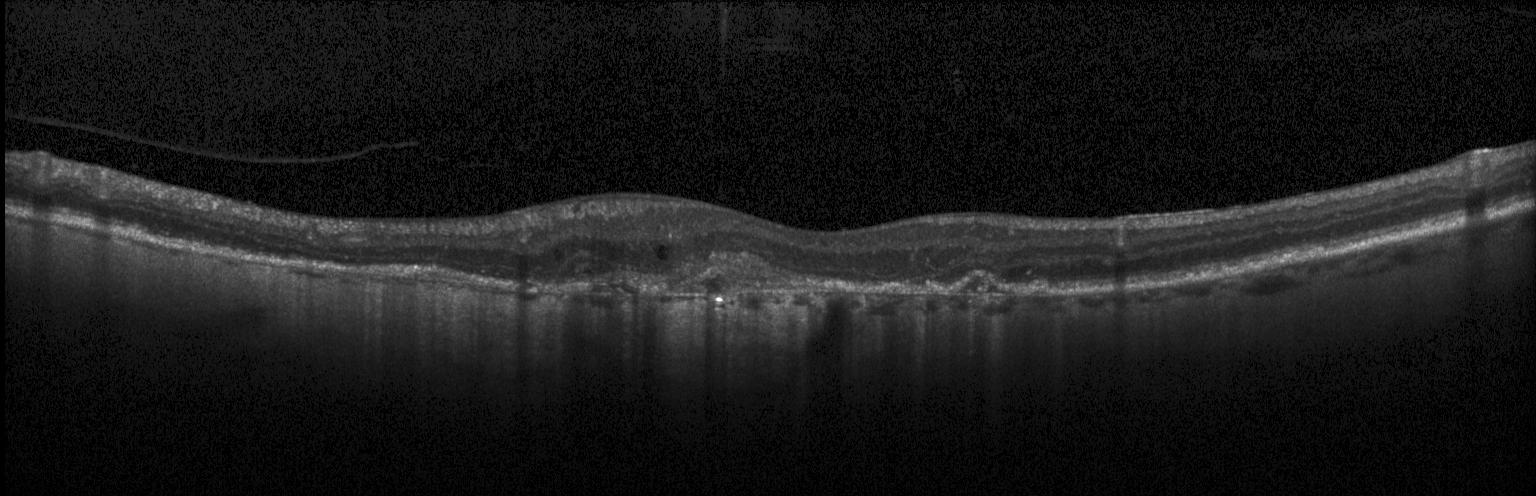

OCT B-scan. Fovea-centered. Spectral-domain OCT. Instrument: Heidelberg Spectralis. Impression: a choroidal neovascular membrane.